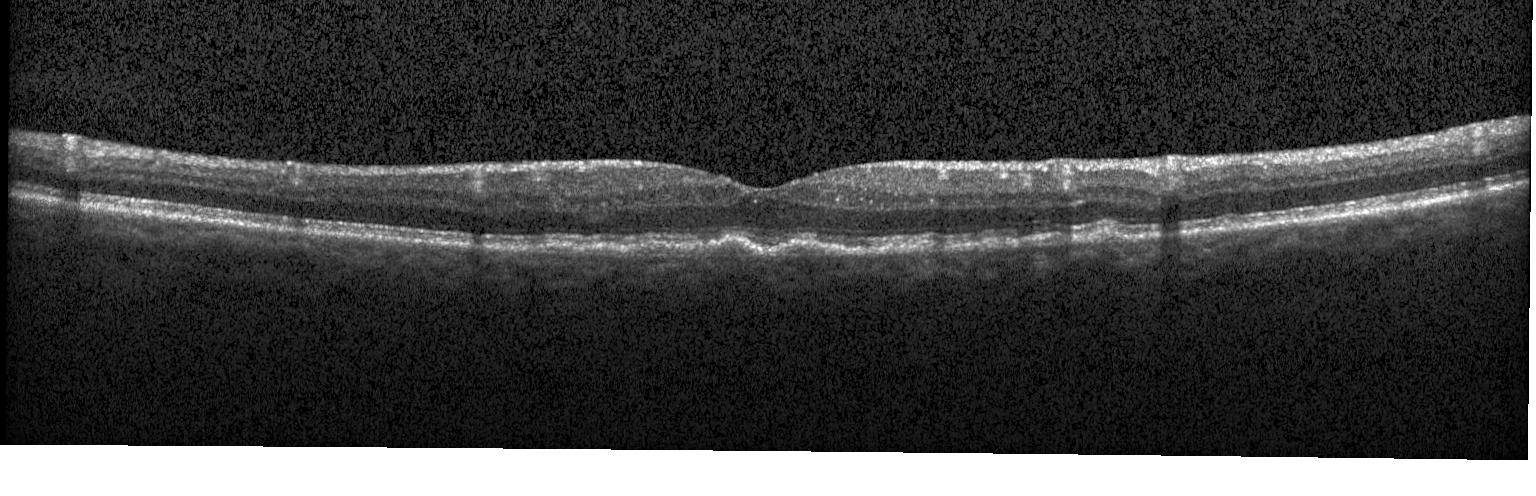
This B-scan demonstrates drusen.